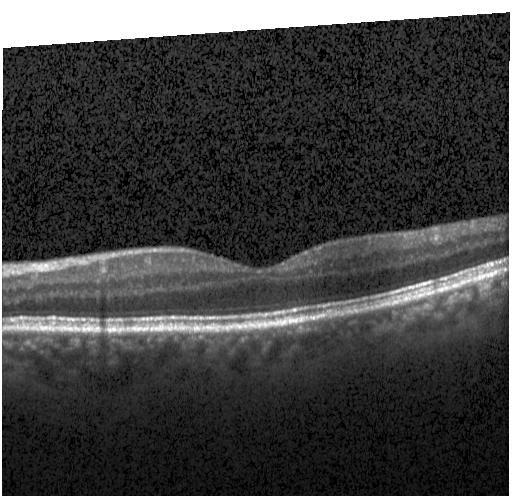
OCT B-scan.
Macular OCT: neither choroidal neovascularization, diabetic macular edema, nor drusen.